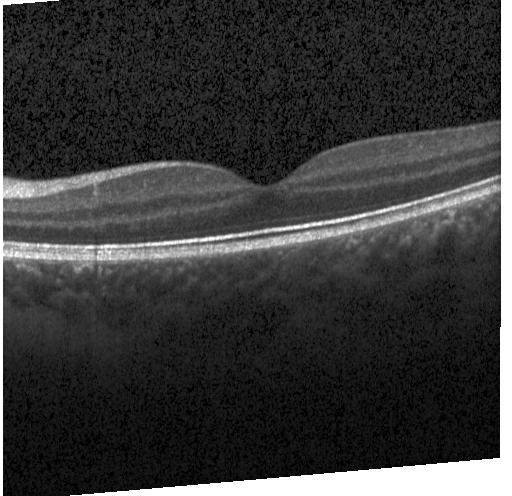
Macular scan; acquired on a Heidelberg Spectralis; retinal OCT cross-section. Diagnosis: no choroidal neovascularization, diabetic macular edema, or drusen.